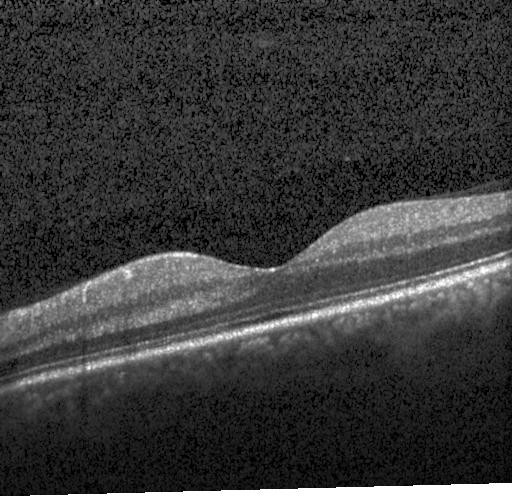
Diagnosis: no CNV, DME, or drusen.